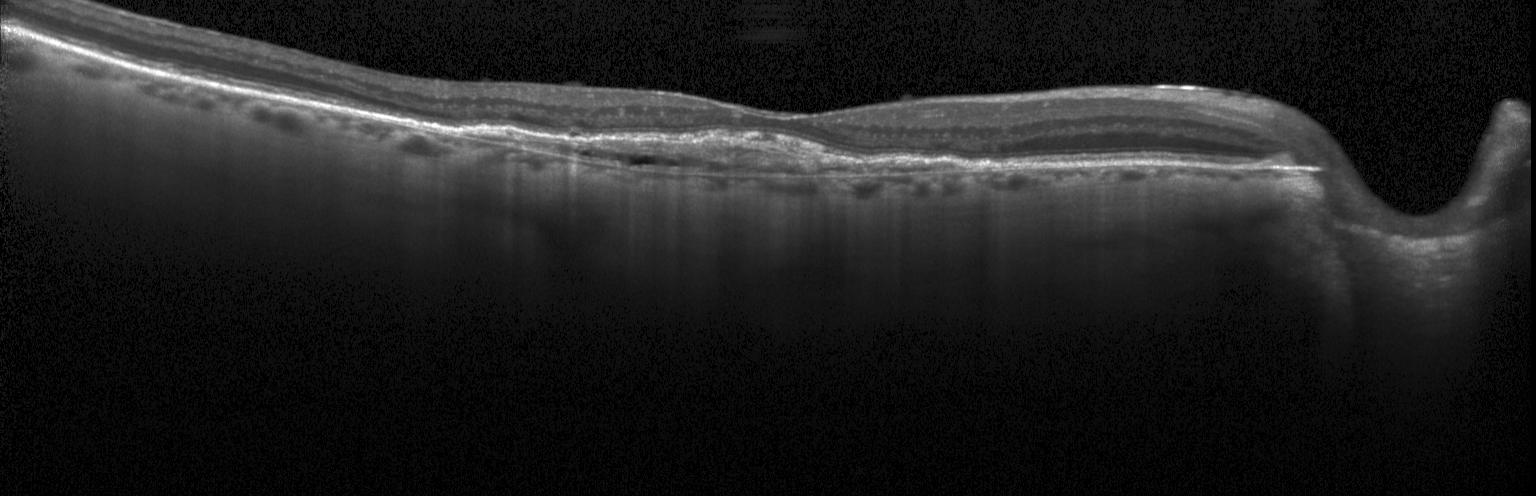

Instrument: Heidelberg Spectralis. OCT line scan. Centered on the fovea. Spectral-domain optical coherence tomography. Impression: a choroidal neovascular membrane.